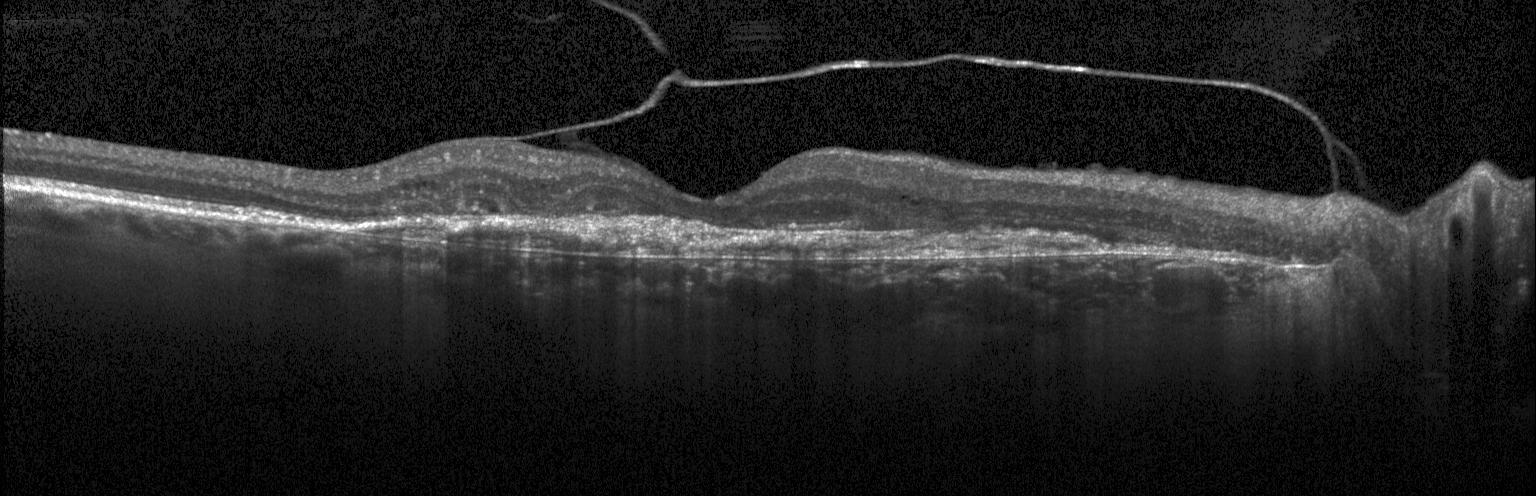 OCT line scan. OCT finding: choroidal neovascularization (CNV).